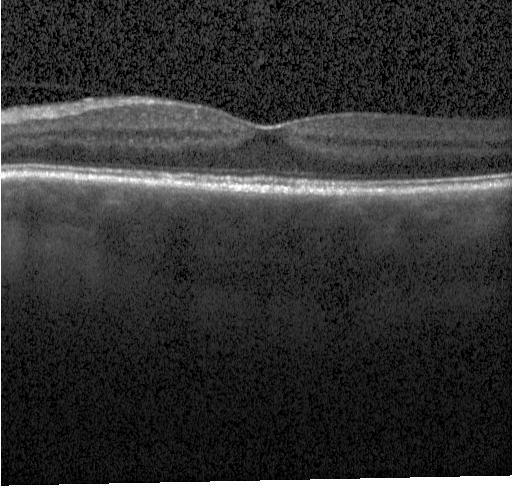 Assessment: no choroidal neovascularization, no diabetic macular edema, and no drusen.